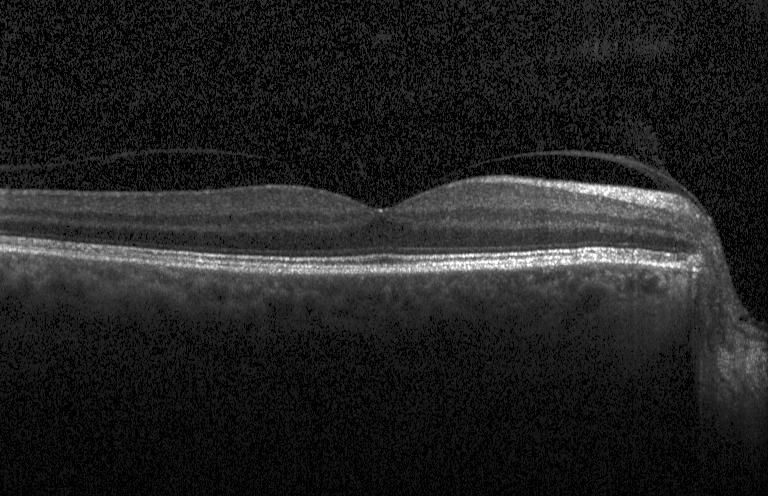

Acquired on a Heidelberg Spectralis, centered on the fovea, spectral-domain optical coherence tomography, OCT line scan.
Finding: no choroidal neovascularization, no diabetic macular edema, and no drusen.